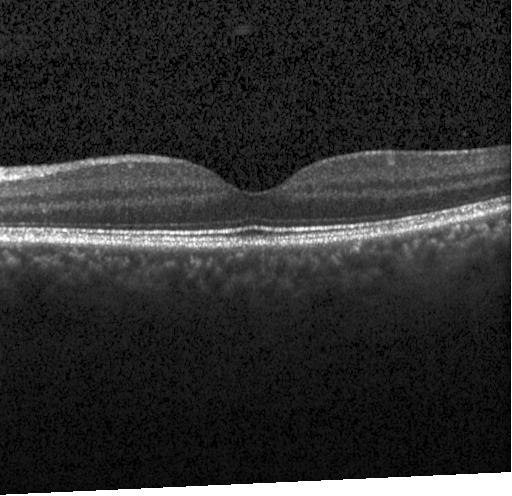
Assessment: no CNV, no DME, and no drusen.